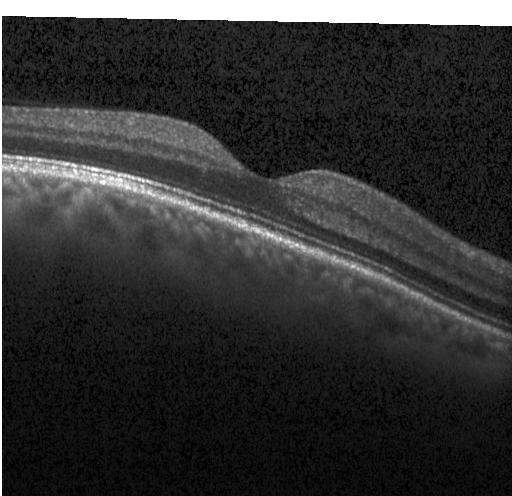 Diagnosis: no CNV, no DME, and no drusen.